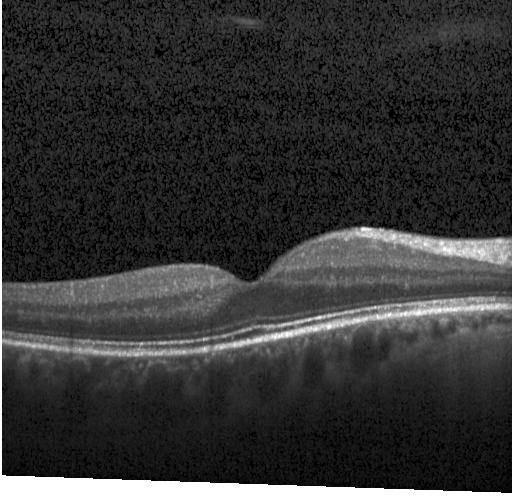 Diagnosis: no CNV, no DME, and no drusen.